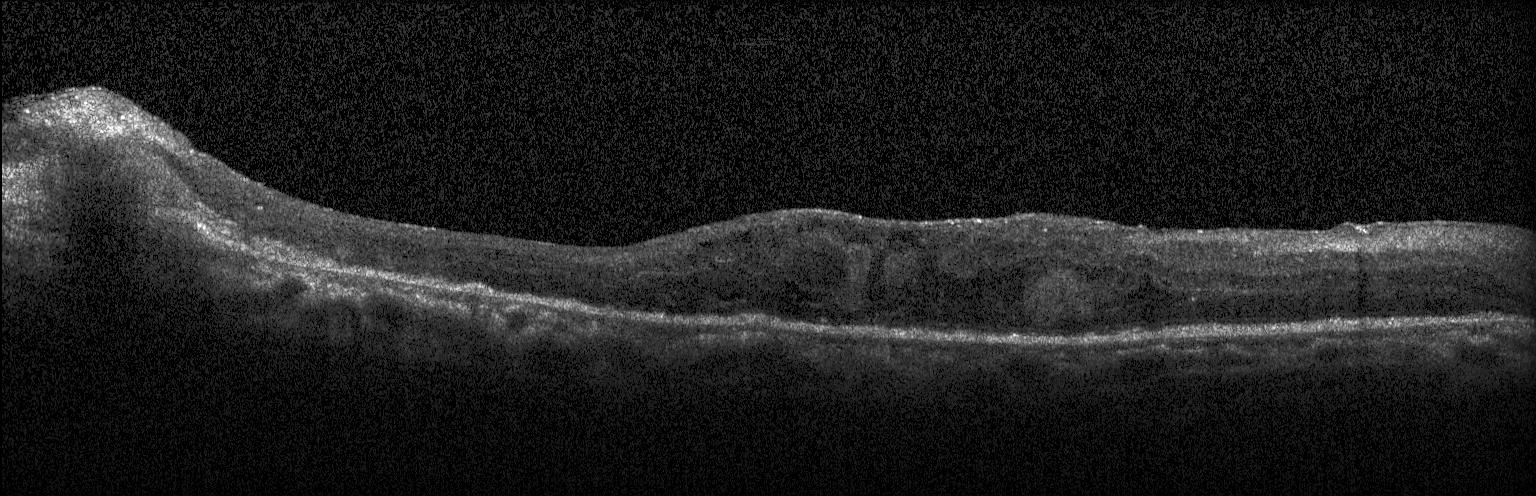

SD-OCT, through the macula, optical coherence tomography scan
Diagnosis: a choroidal neovascular membrane.